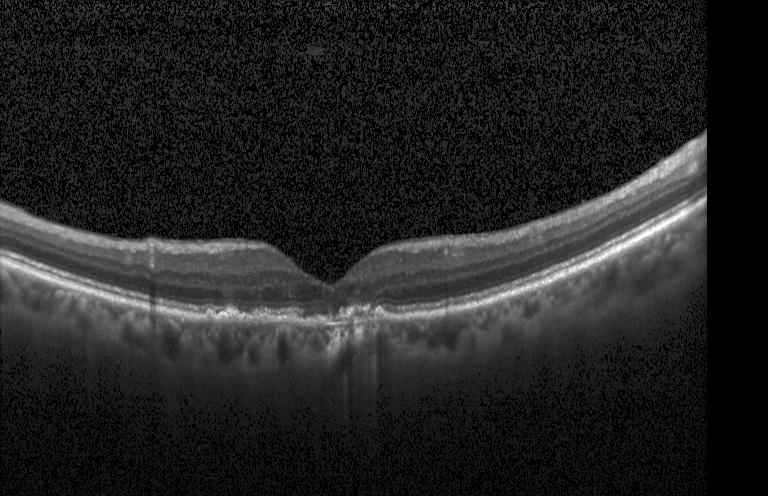
Retinal OCT B-scan. Spectral-domain OCT.
Choroidal neovascularization (CNV).